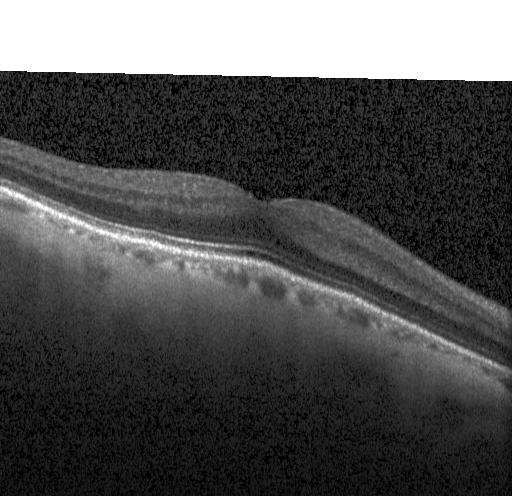

The scan shows no choroidal neovascularization, no diabetic macular edema, and no drusen.